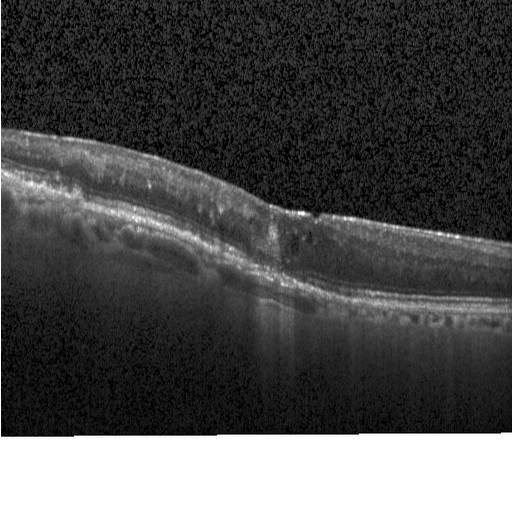 Instrument: Heidelberg Spectralis; fovea-centered; optical coherence tomography B-scan; spectral-domain OCT.
Impression: DME.